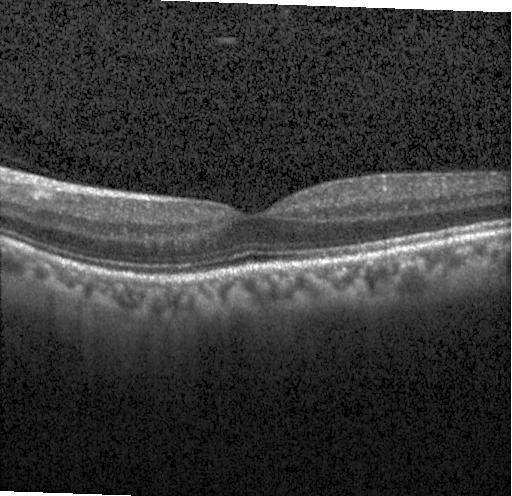 Retinal OCT cross-section.
Finding: no CNV, DME, or drusen.